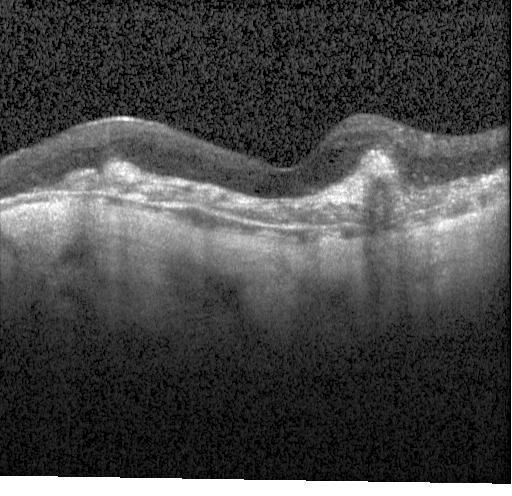 Macular scan · Heidelberg Spectralis OCT system · spectral-domain OCT · retinal OCT B-scan
A choroidal neovascular membrane.